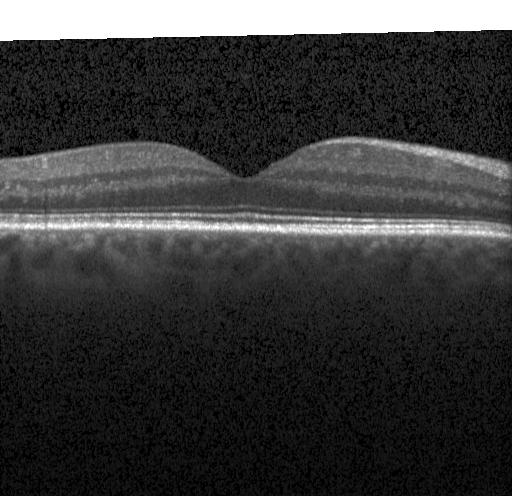
Neither CNV, DME, nor drusen.